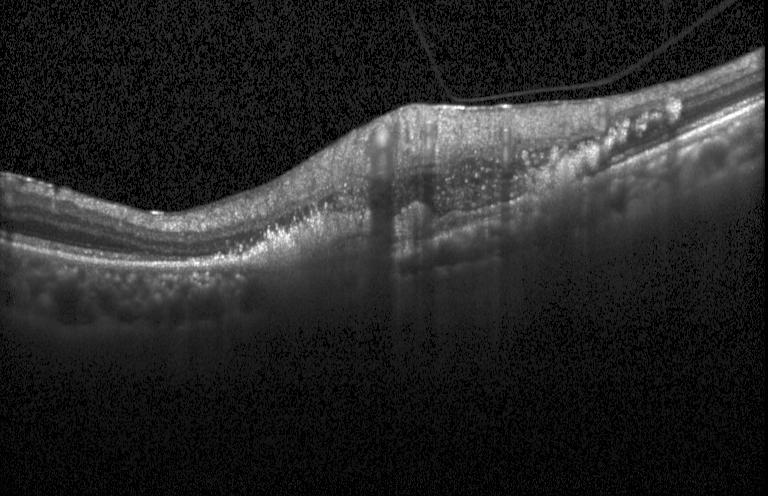
Fovea-centered. Retinal OCT B-scan. Instrument: Heidelberg Spectralis. Spectral-domain OCT. Impression: a choroidal neovascular membrane.